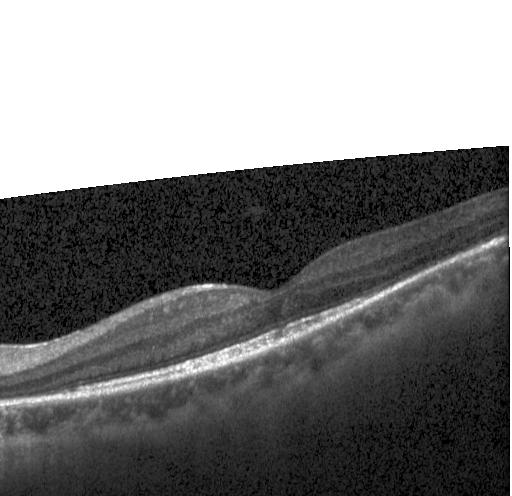

The scan shows no choroidal neovascularization, no diabetic macular edema, and no drusen.